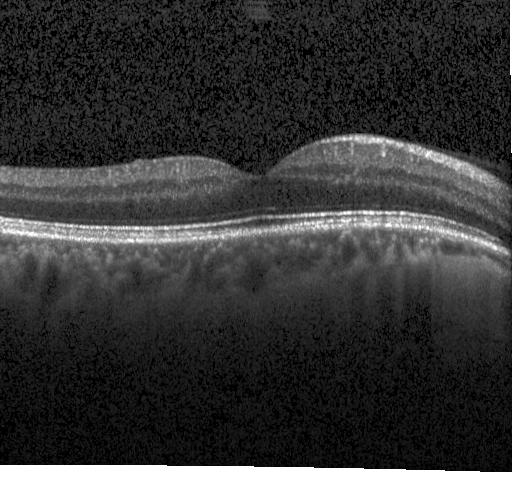 Impression: no CNV, DME, or drusen.